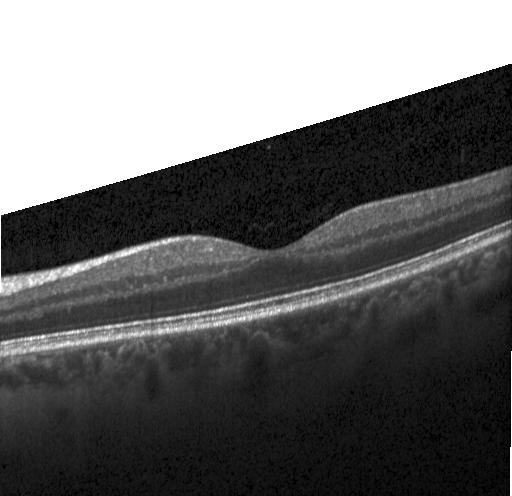

Diagnosis: no choroidal neovascularization, diabetic macular edema, or drusen.